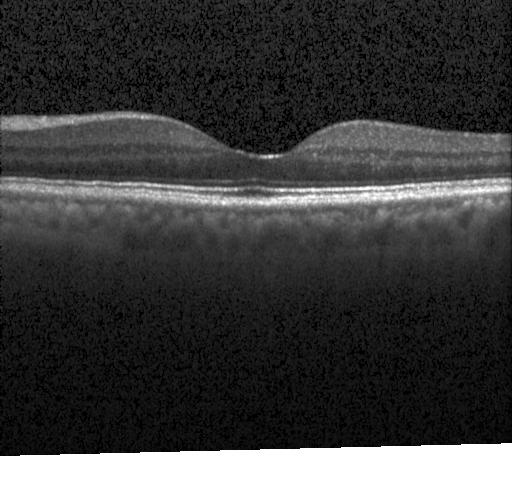
Heidelberg Spectralis OCT system. SD-OCT. Optical coherence tomography B-scan. Impression: neither choroidal neovascularization, diabetic macular edema, nor drusen.